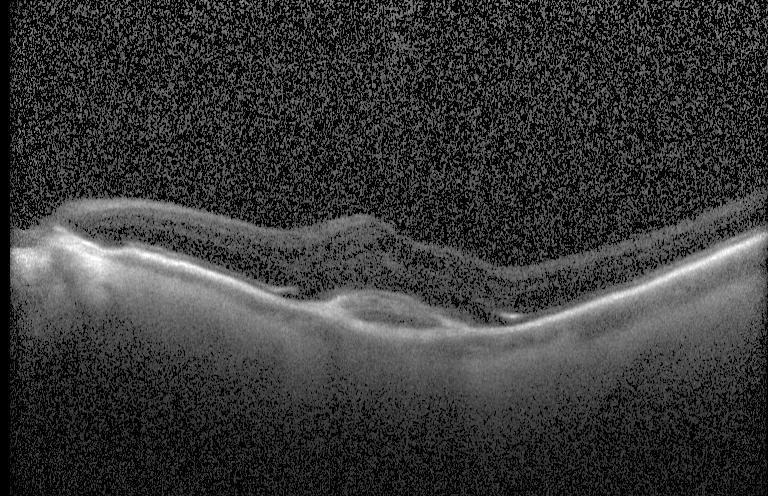 OCT B-scan — Assessment: CNV.